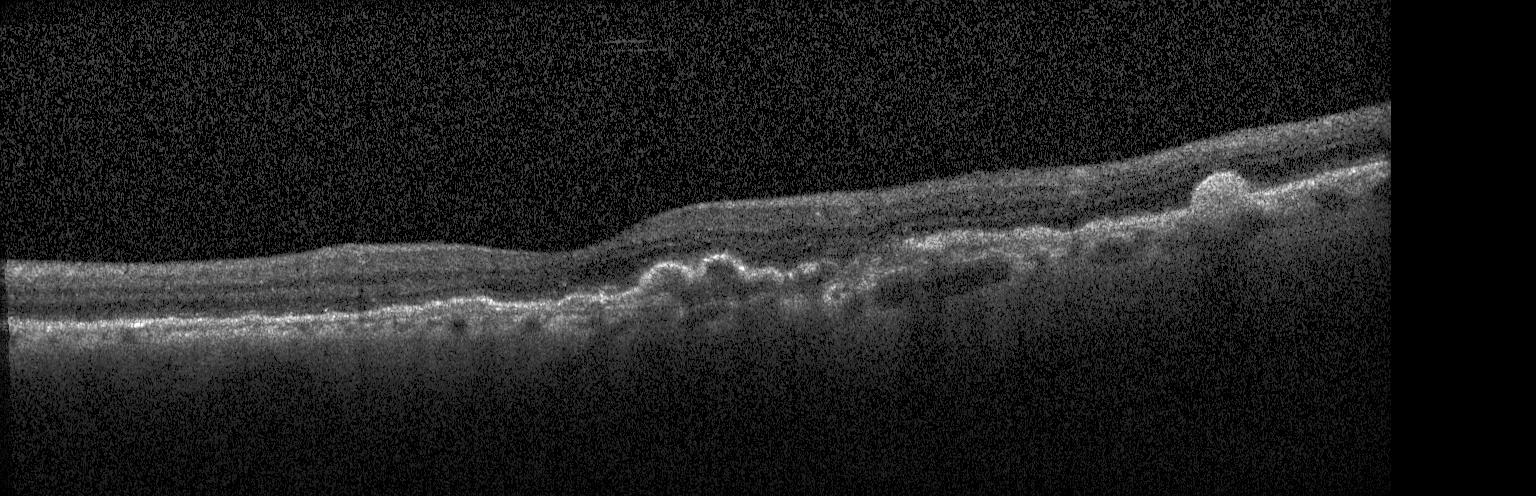 Impression: a choroidal neovascular membrane.